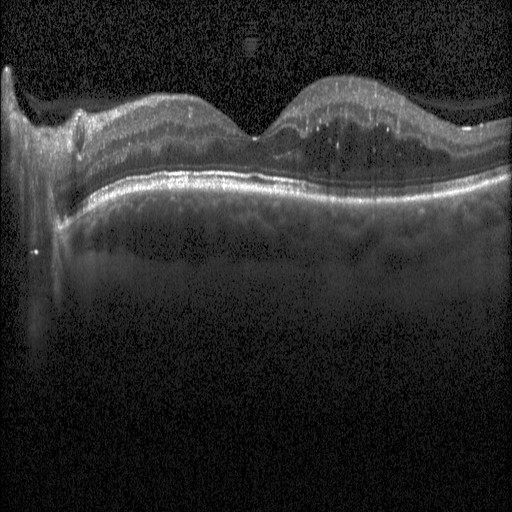

OCT B-scan showing DME.